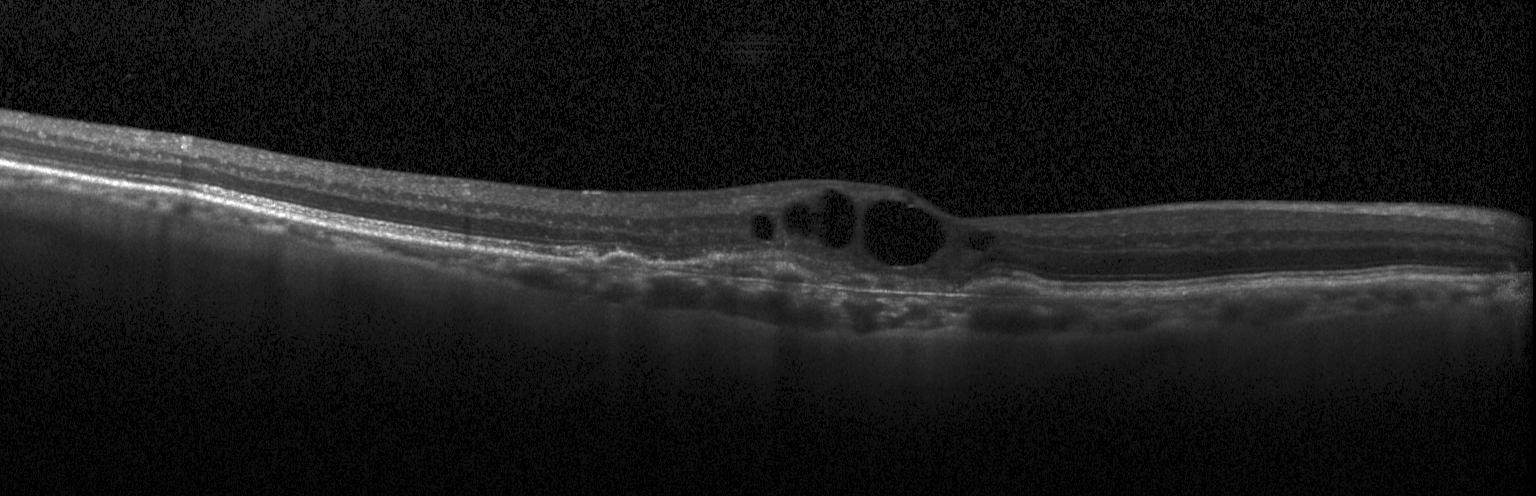 Fovea-centered, Heidelberg Spectralis OCT system, retinal OCT B-scan
This B-scan demonstrates choroidal neovascularization.